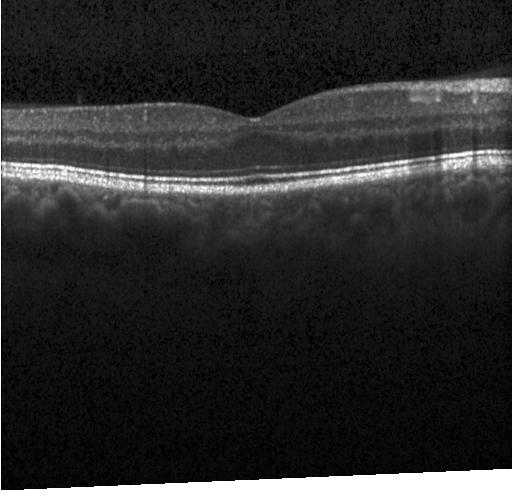

SD-OCT · through the macula · instrument: Heidelberg Spectralis · retinal OCT B-scan. No choroidal neovascularization, no diabetic macular edema, and no drusen.